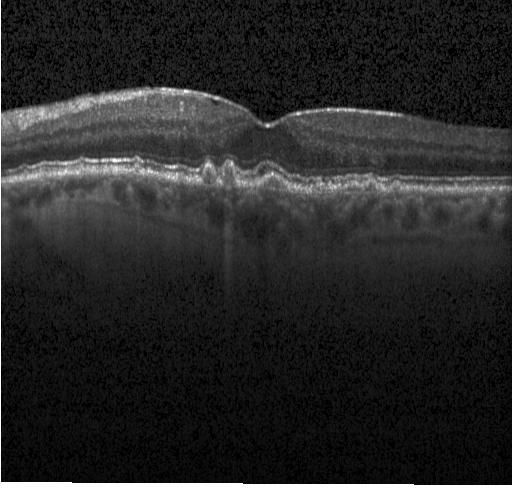
Finding: sub-RPE drusenoid deposits.